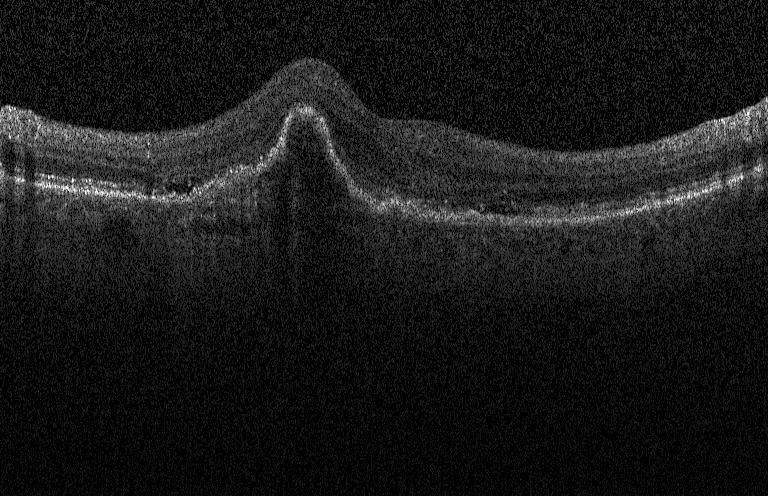 Impression: choroidal neovascularization (CNV).